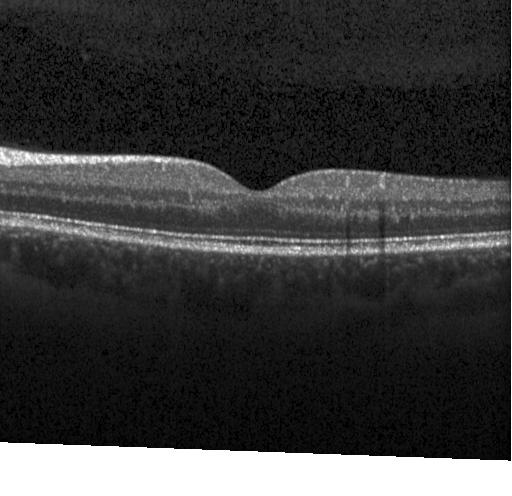
Retinal OCT cross-section
Assessment: no choroidal neovascularization, no diabetic macular edema, and no drusen.